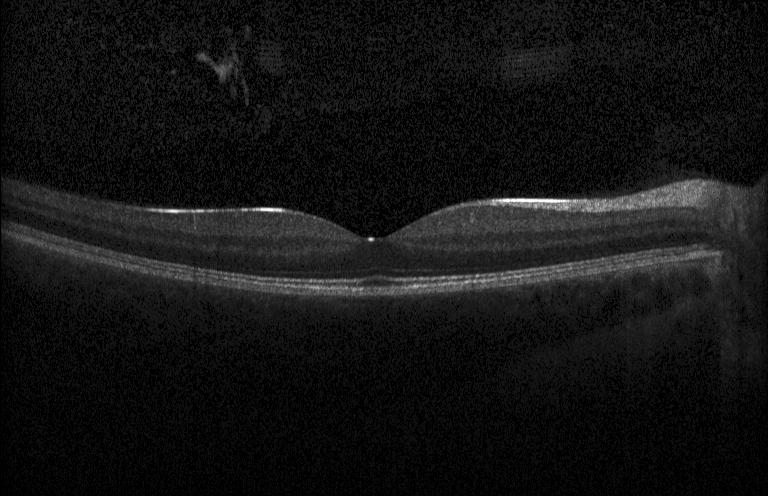

Finding: neither choroidal neovascularization, diabetic macular edema, nor drusen.